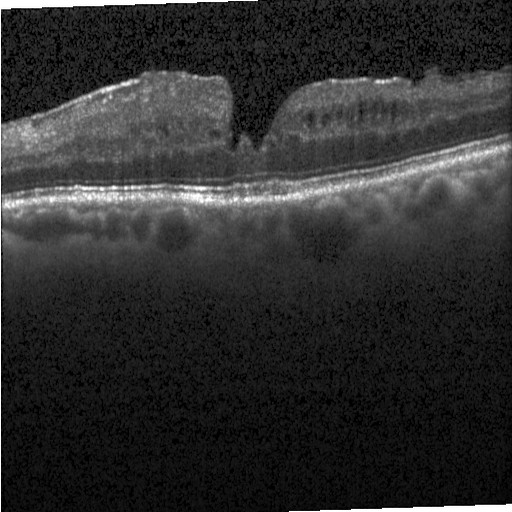 Retinal OCT cross-section
Finding: DME.